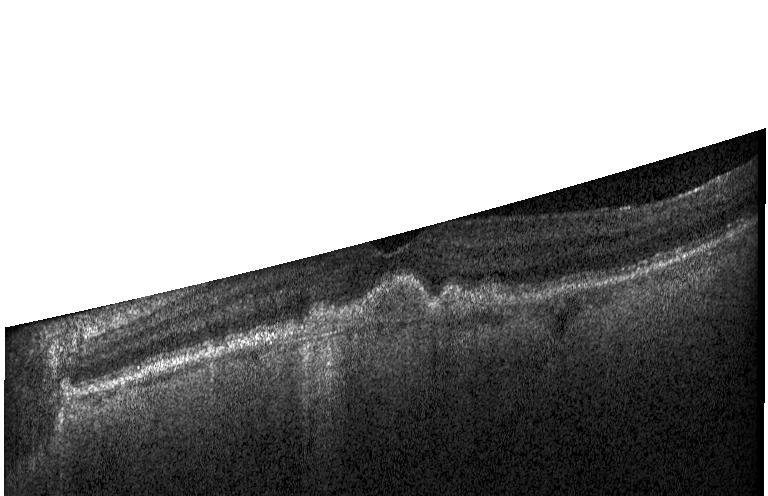 SD-OCT; retinal OCT B-scan; fovea-centered — OCT finding: a choroidal neovascular membrane.